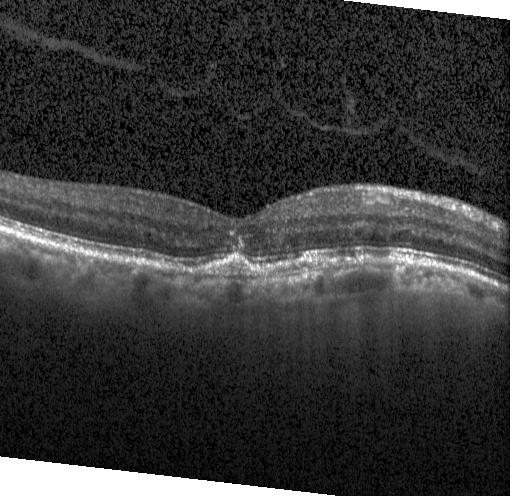
Macular OCT demonstrating a choroidal neovascular membrane.